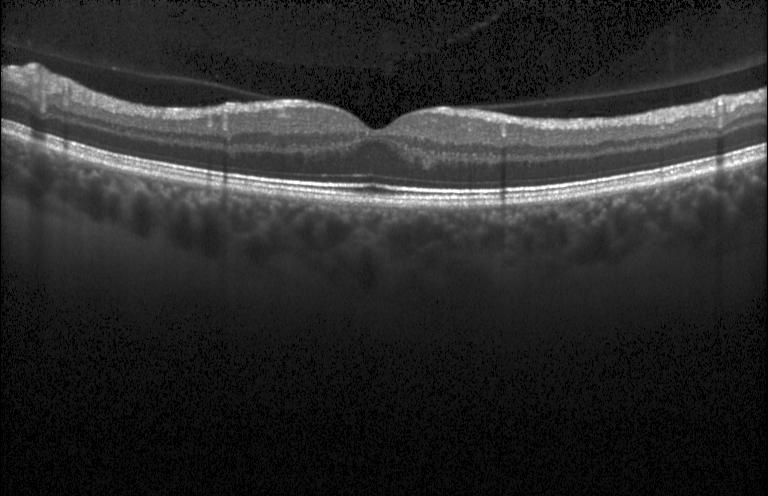

Retinal OCT cross-section · centered on the fovea · Heidelberg Spectralis.
Finding: no evidence of choroidal neovascularization, diabetic macular edema, or drusen.